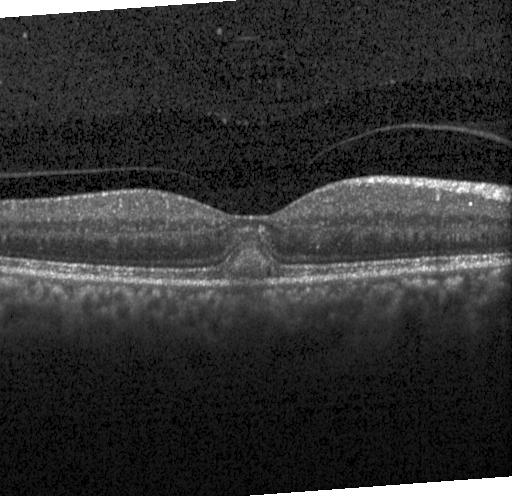
Impression: CNV.